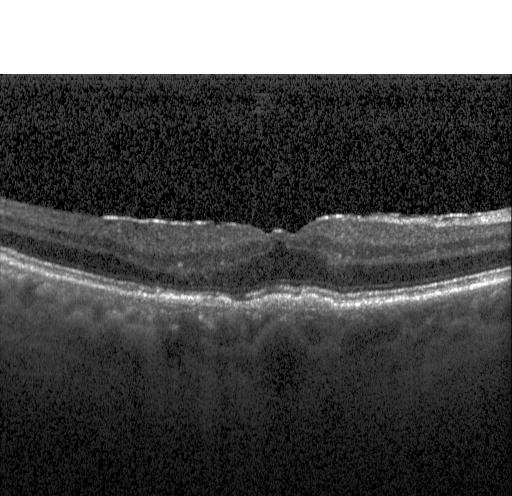
Acquired on a Heidelberg Spectralis, retinal OCT cross-section, SD-OCT, through the macula.
Impression: a choroidal neovascular membrane.